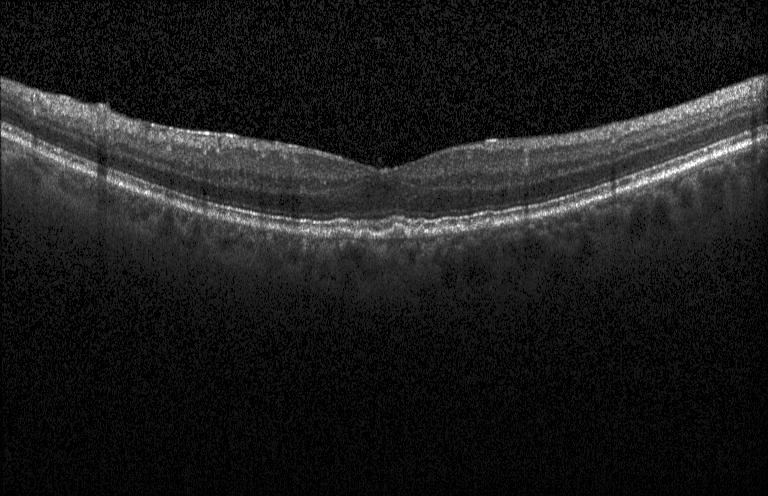

Dx: multiple drusen.